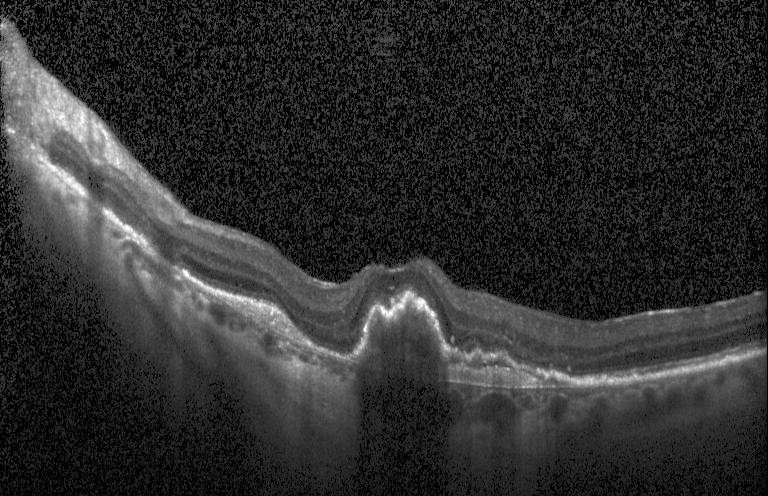 Instrument: Heidelberg Spectralis. Spectral-domain OCT. Retinal OCT cross-section. Through the macula. Finding: a choroidal neovascular membrane.